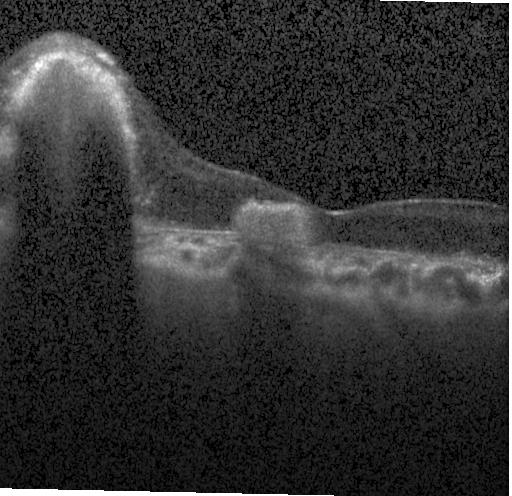

Optical coherence tomography scan. Macular scan.
Impression: choroidal neovascularization (CNV).